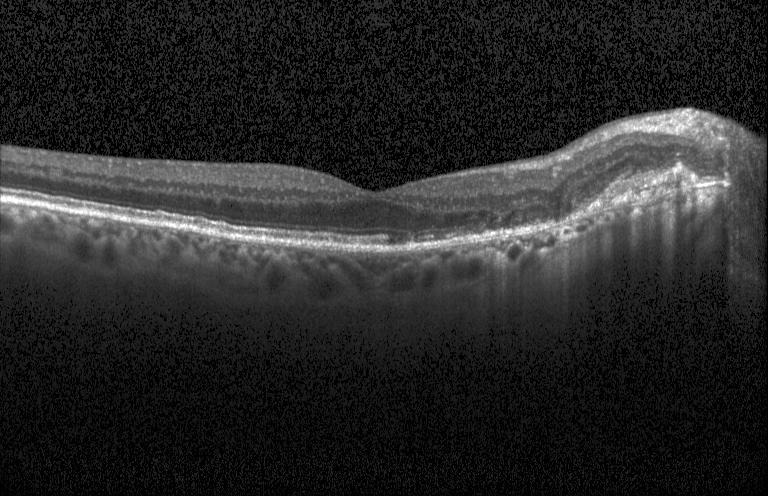

Horizontal scan through the fovea; Heidelberg Spectralis; retinal OCT B-scan. This B-scan demonstrates choroidal neovascularization (CNV).